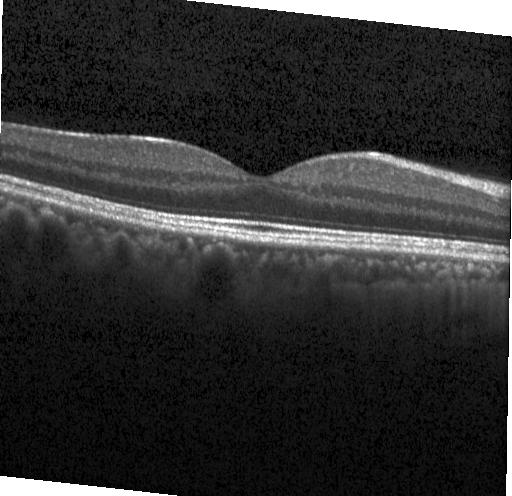
OCT finding: neither CNV, DME, nor drusen.